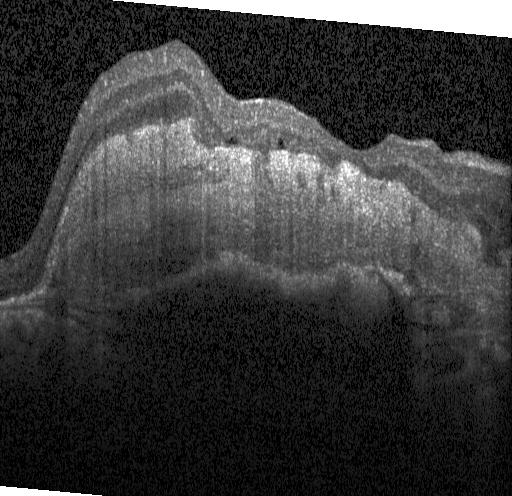 Optical coherence tomography B-scan, Heidelberg Spectralis, through the macula
Finding: choroidal neovascularization.